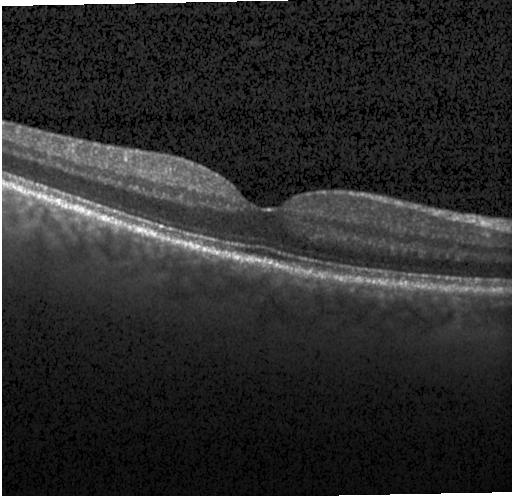

OCT B-scan. OCT finding: no CNV, no DME, and no drusen.